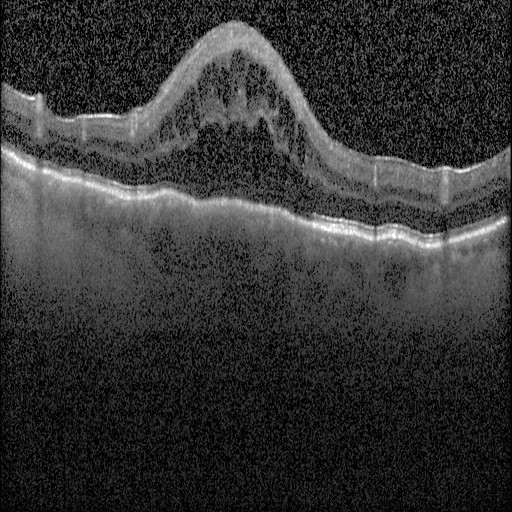 Retinal OCT B-scan. Heidelberg Spectralis OCT system
Impression: diabetic macular edema.